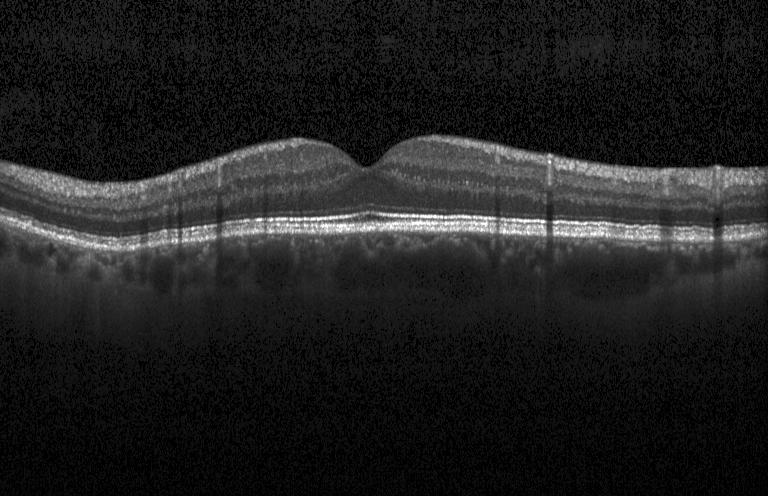
Through the macula · OCT B-scan · Heidelberg Spectralis — Finding: no evidence of choroidal neovascularization, diabetic macular edema, or drusen.